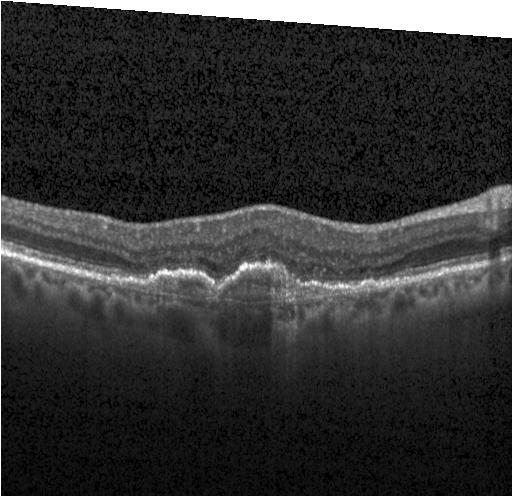
Retinal OCT B-scan. The scan shows a choroidal neovascular membrane.